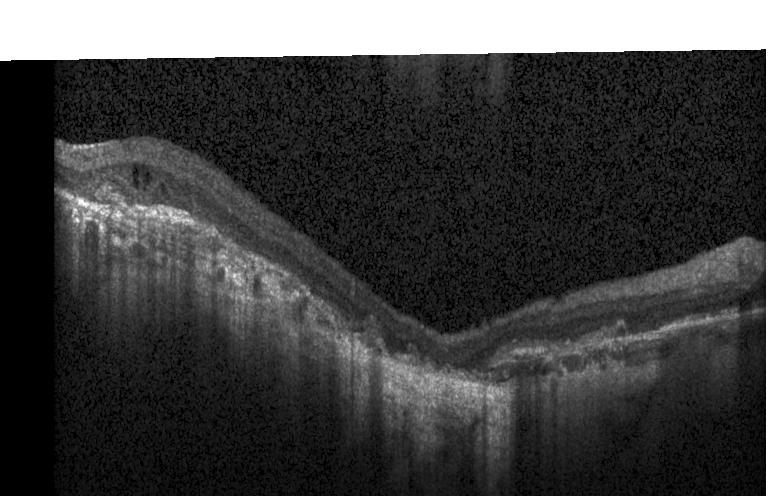 Spectral-domain OCT B-scan: a choroidal neovascular membrane.